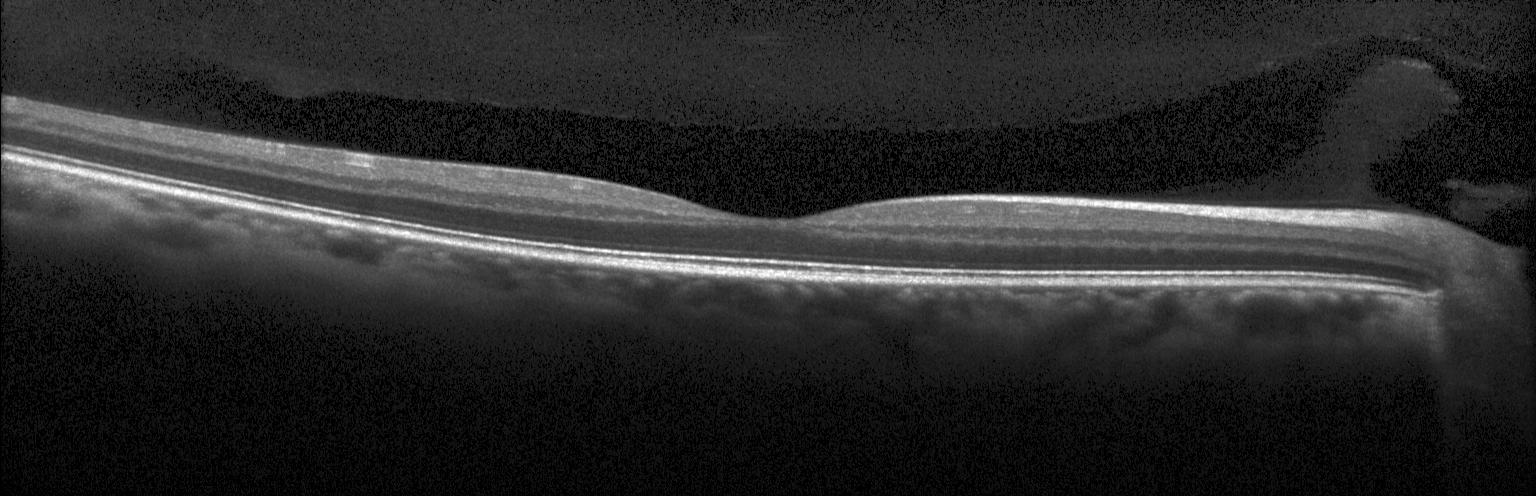

Acquired on a Heidelberg Spectralis · retinal OCT B-scan.
No choroidal neovascularization, diabetic macular edema, or drusen.